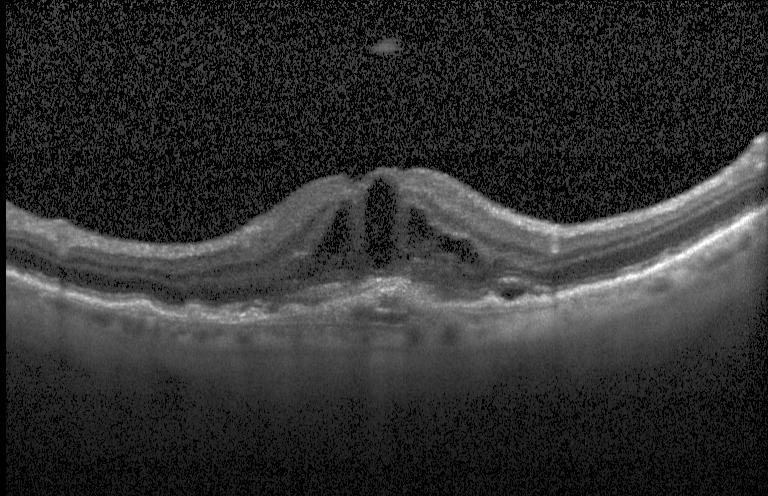

OCT scan showing choroidal neovascularization (CNV).